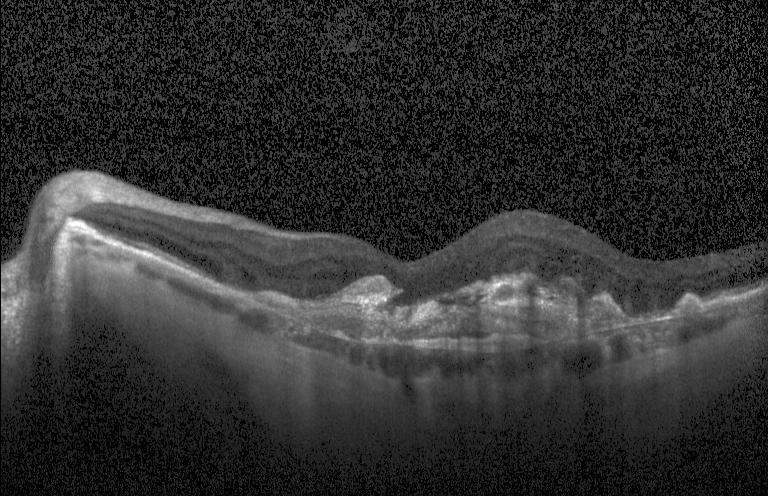 Impression: choroidal neovascularization.